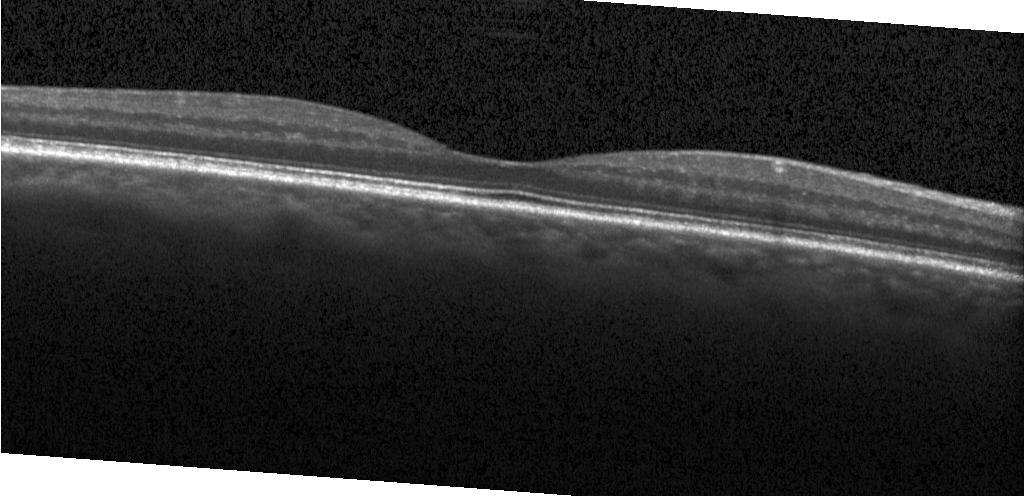

OCT finding: no evidence of choroidal neovascularization, diabetic macular edema, or drusen.